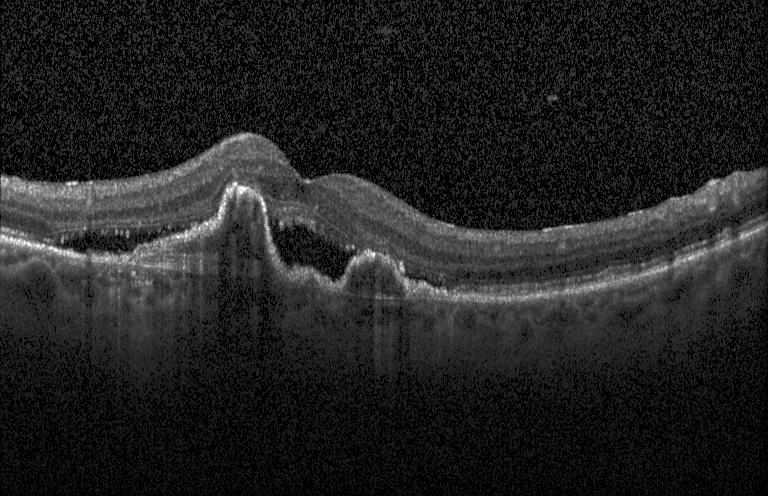

Spectral-domain OCT B-scan: CNV.